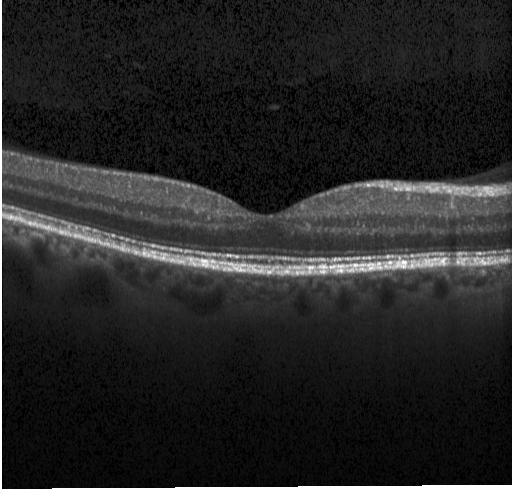
Optical coherence tomography scan · through the macula · Heidelberg Spectralis — Macular OCT: neither CNV, DME, nor drusen.